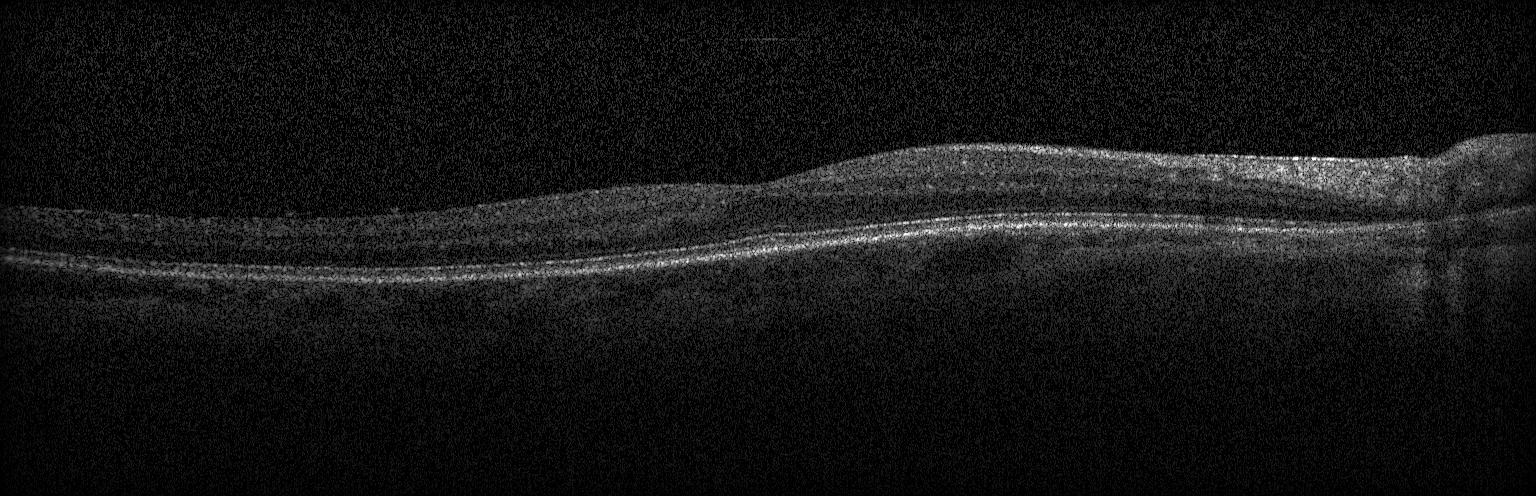 Centered on the fovea · OCT line scan · Heidelberg Spectralis · spectral-domain optical coherence tomography.
Impression: no evidence of choroidal neovascularization, diabetic macular edema, or drusen.